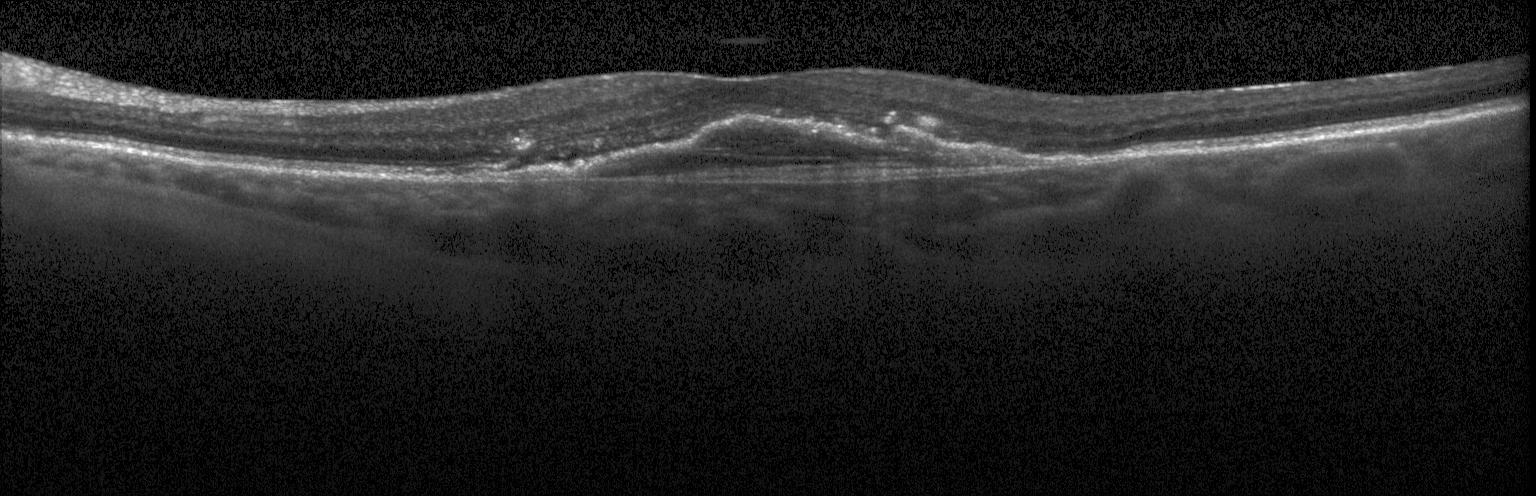

Retinal OCT cross-section
A choroidal neovascular membrane.